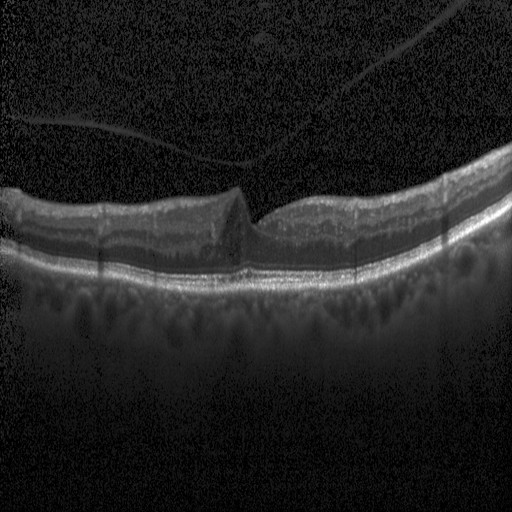

Spectral-domain optical coherence tomography. Instrument: Heidelberg Spectralis. Through the macula. Optical coherence tomography scan — Finding: DME.